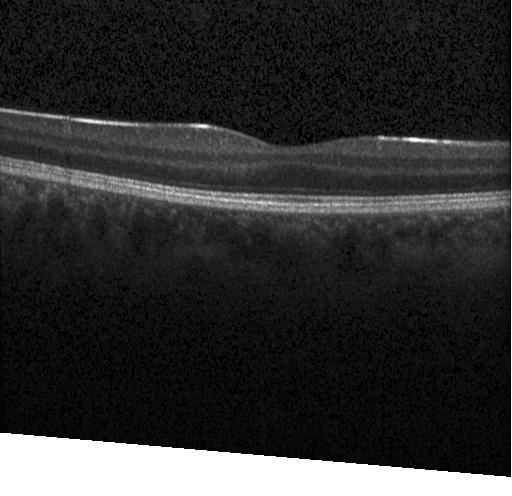

SD-OCT; retinal OCT B-scan; fovea-centered; Heidelberg Spectralis. Dx: no choroidal neovascularization, diabetic macular edema, or drusen.